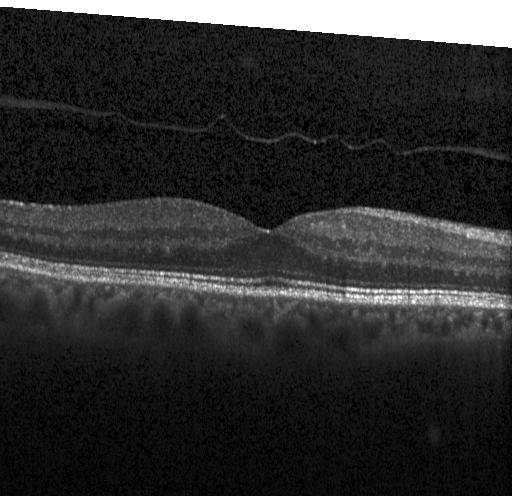

Spectral-domain optical coherence tomography · retinal OCT B-scan · Heidelberg Spectralis.
Finding: no CNV, DME, or drusen.